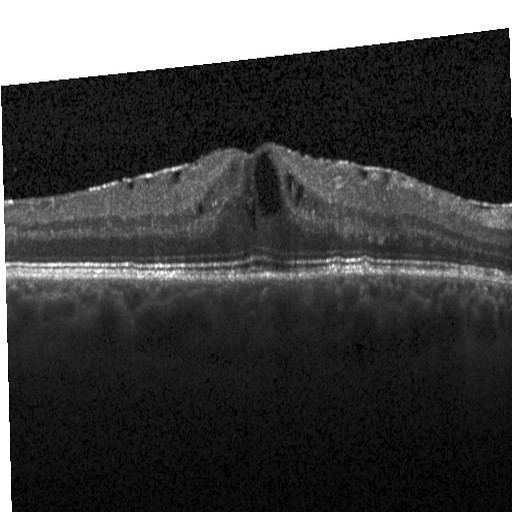

Dx: diabetic macular edema (DME).